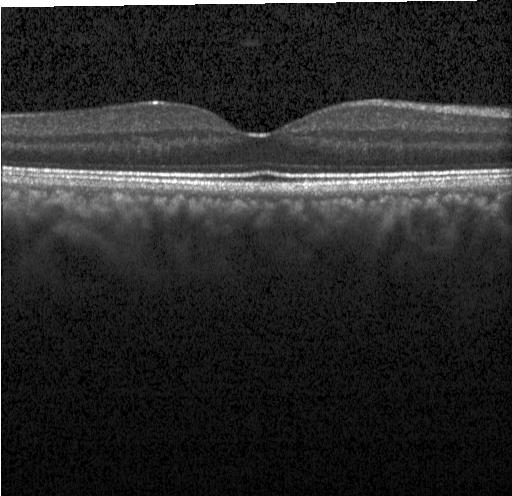
No evidence of choroidal neovascularization, diabetic macular edema, or drusen.